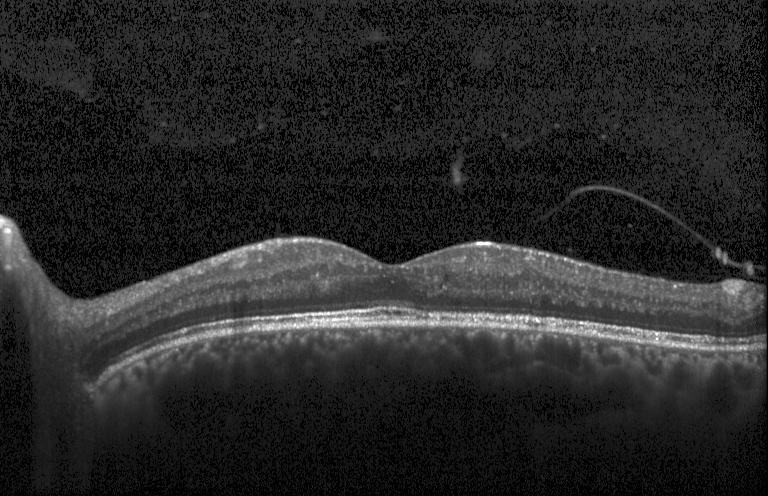 Optical coherence tomography scan — Finding: no choroidal neovascularization, no diabetic macular edema, and no drusen.